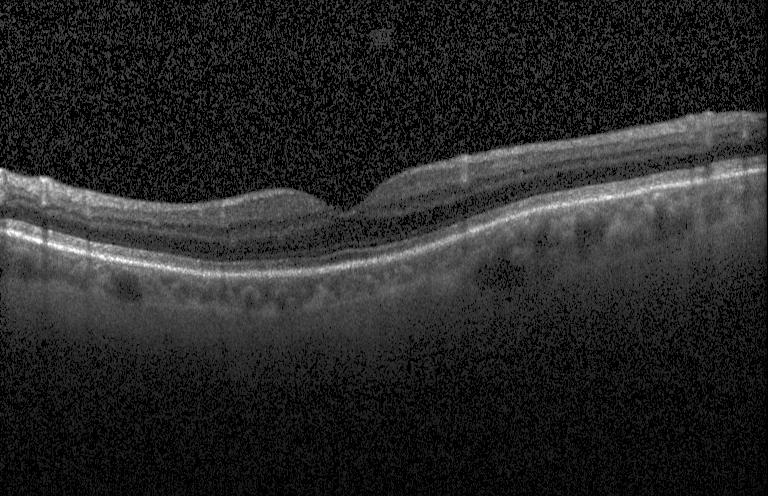

Impression: no evidence of choroidal neovascularization, diabetic macular edema, or drusen.